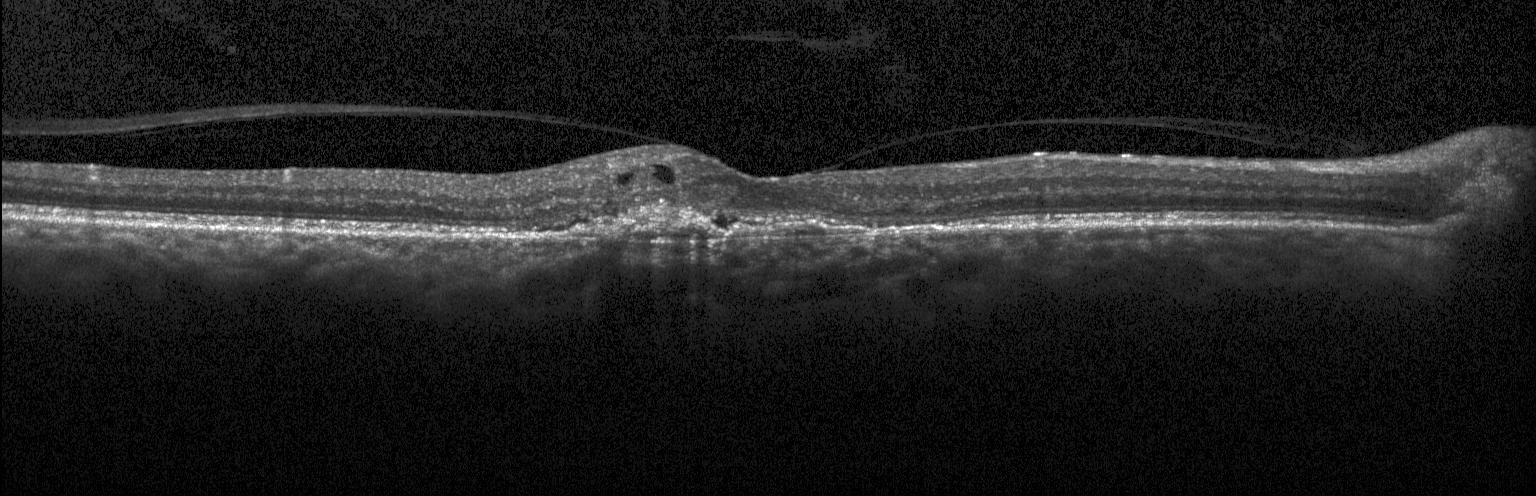 Macular OCT demonstrating a choroidal neovascular membrane.